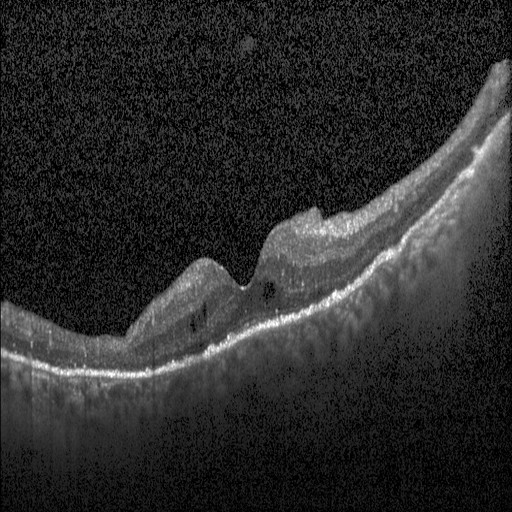 Macular OCT demonstrating DME.